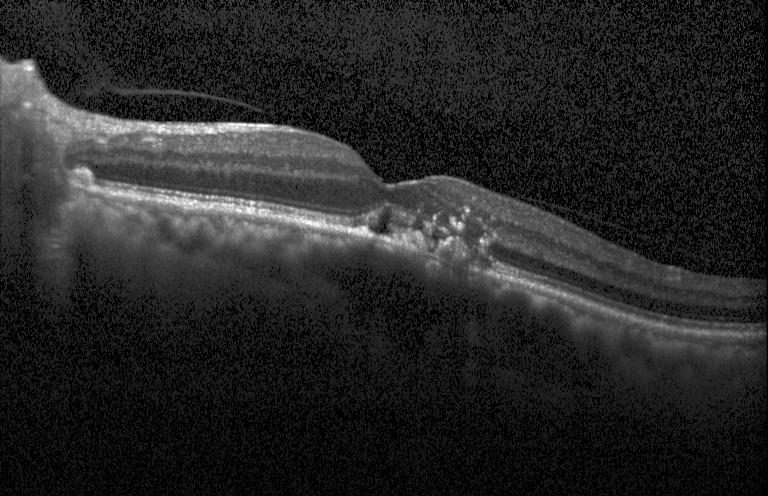

Optical coherence tomography scan, macular scan, Heidelberg Spectralis — Choroidal neovascularization (CNV).